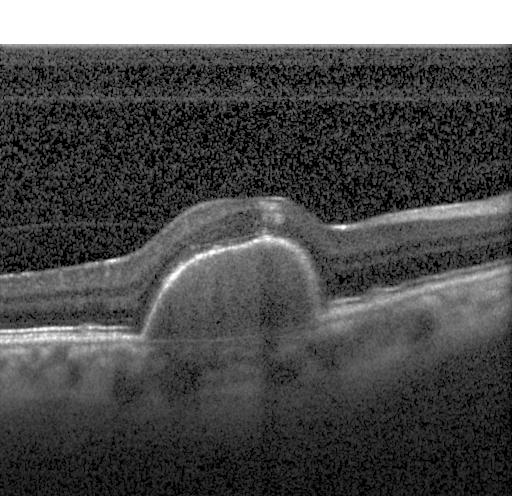
Optical coherence tomography B-scan.
Choroidal neovascularization (CNV).